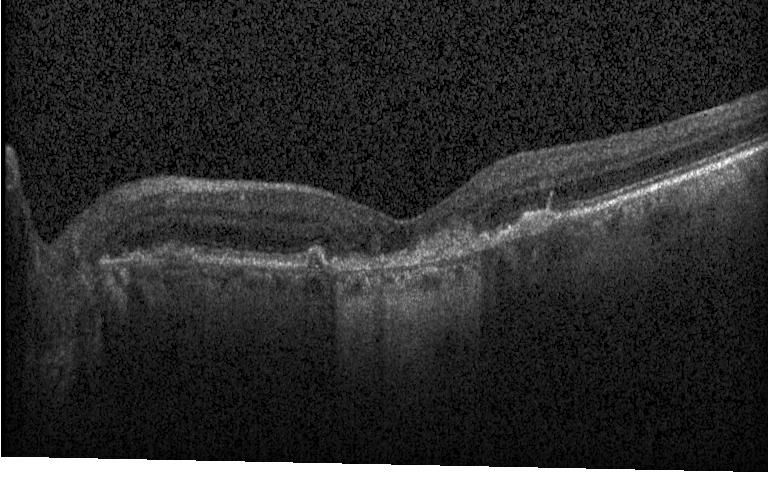

OCT finding: CNV.